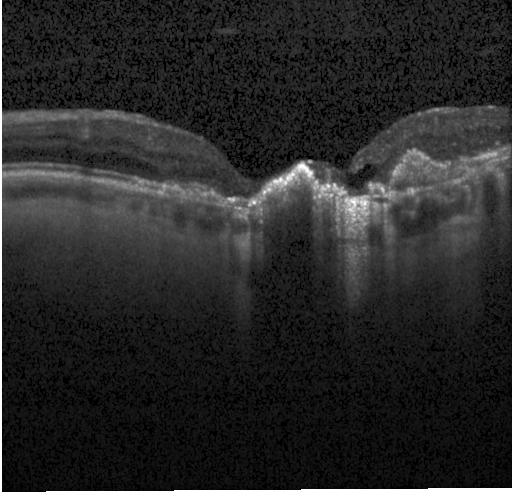

Centered on the fovea, instrument: Heidelberg Spectralis, spectral-domain OCT, retinal OCT cross-section.
This B-scan demonstrates a choroidal neovascular membrane.